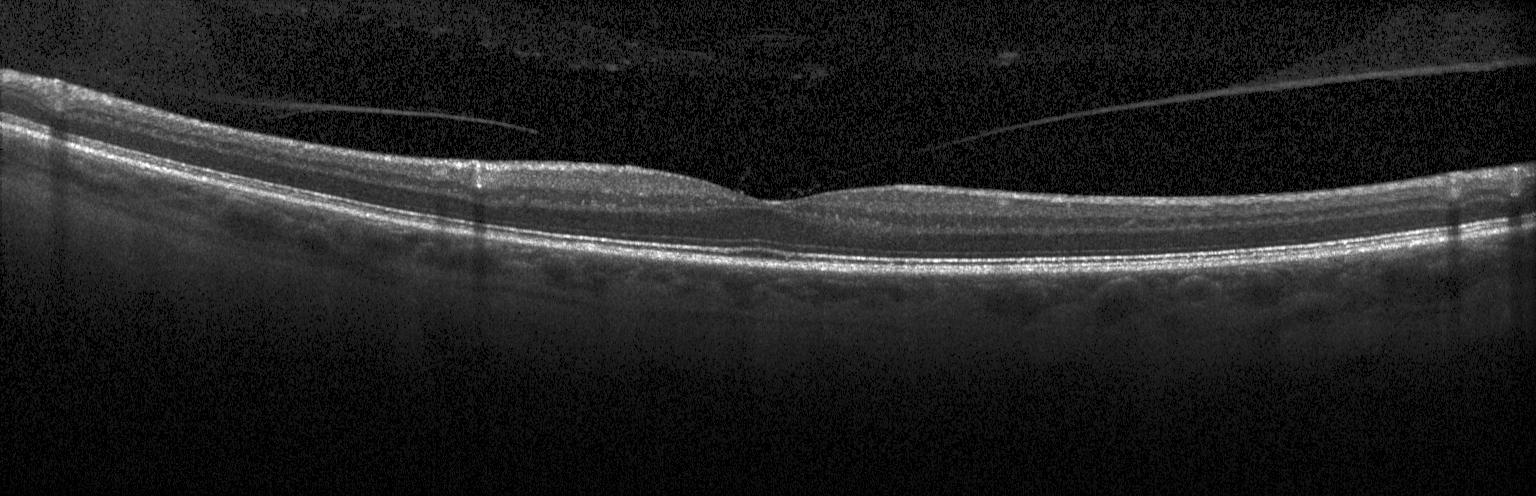

OCT line scan — Assessment: no evidence of CNV, DME, or drusen.